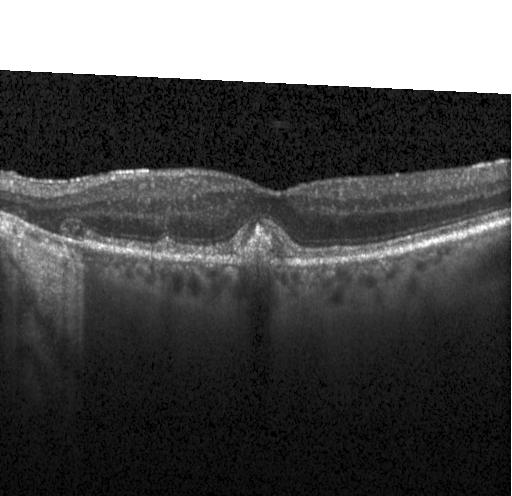

Finding: choroidal neovascularization (CNV).